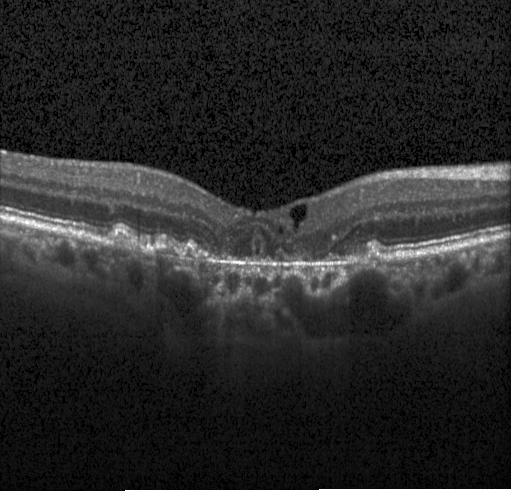
Acquired on a Heidelberg Spectralis; SD-OCT; optical coherence tomography B-scan; centered on the fovea — This B-scan demonstrates a choroidal neovascular membrane.